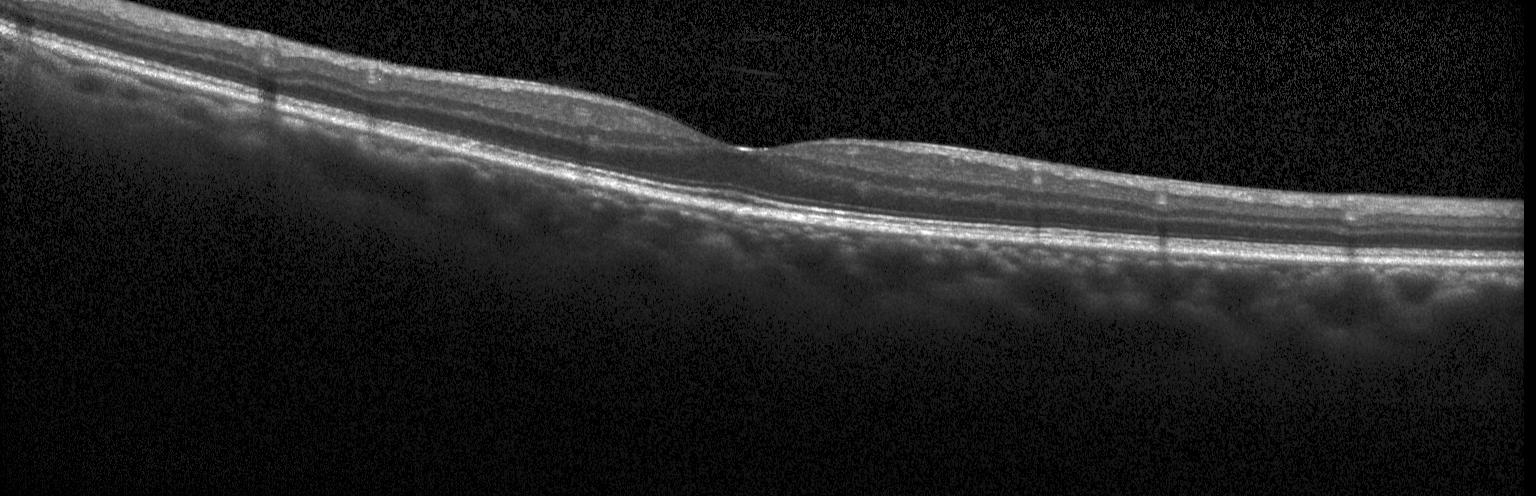
Through the macula; spectral-domain optical coherence tomography; Heidelberg Spectralis OCT system; optical coherence tomography B-scan
This B-scan demonstrates no choroidal neovascularization, no diabetic macular edema, and no drusen.